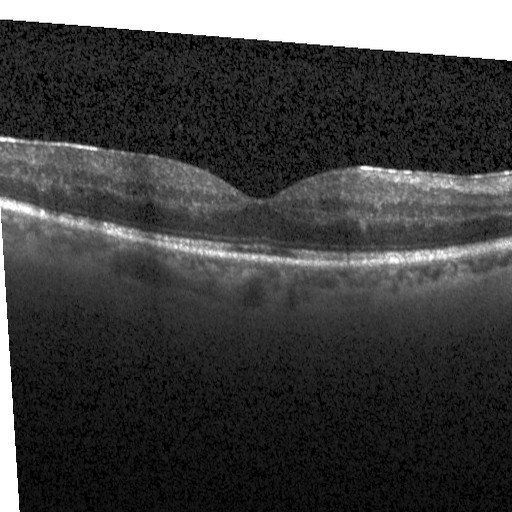
Retinal OCT B-scan; spectral-domain optical coherence tomography; through the macula; Heidelberg Spectralis OCT system.
This B-scan demonstrates diabetic macular edema (DME).